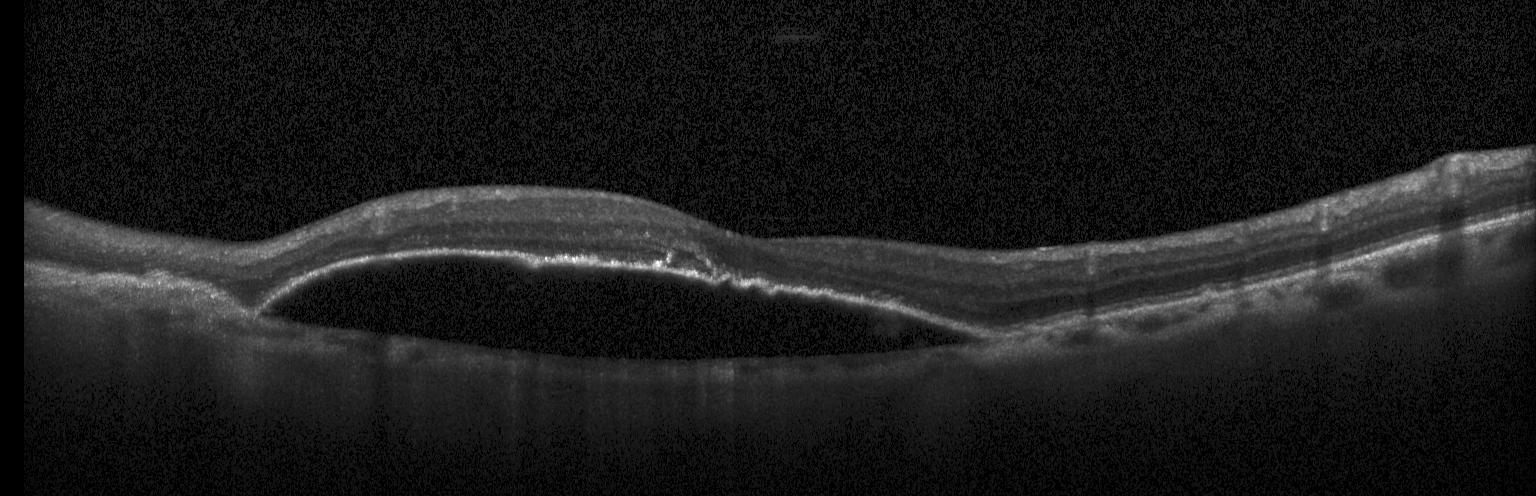

OCT line scan. Acquired on a Heidelberg Spectralis. Centered on the fovea. SD-OCT. Finding: choroidal neovascularization.